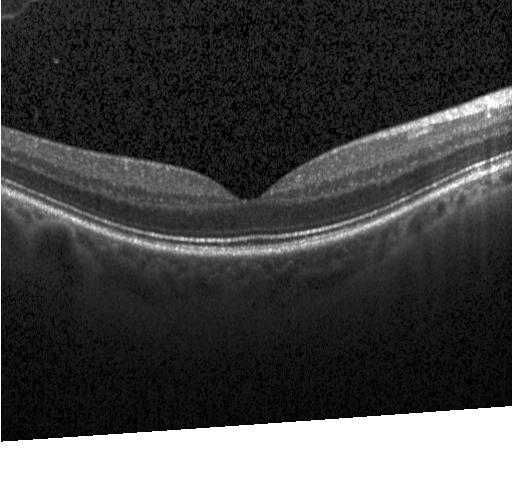 Retinal OCT cross-section showing no evidence of CNV, DME, or drusen.